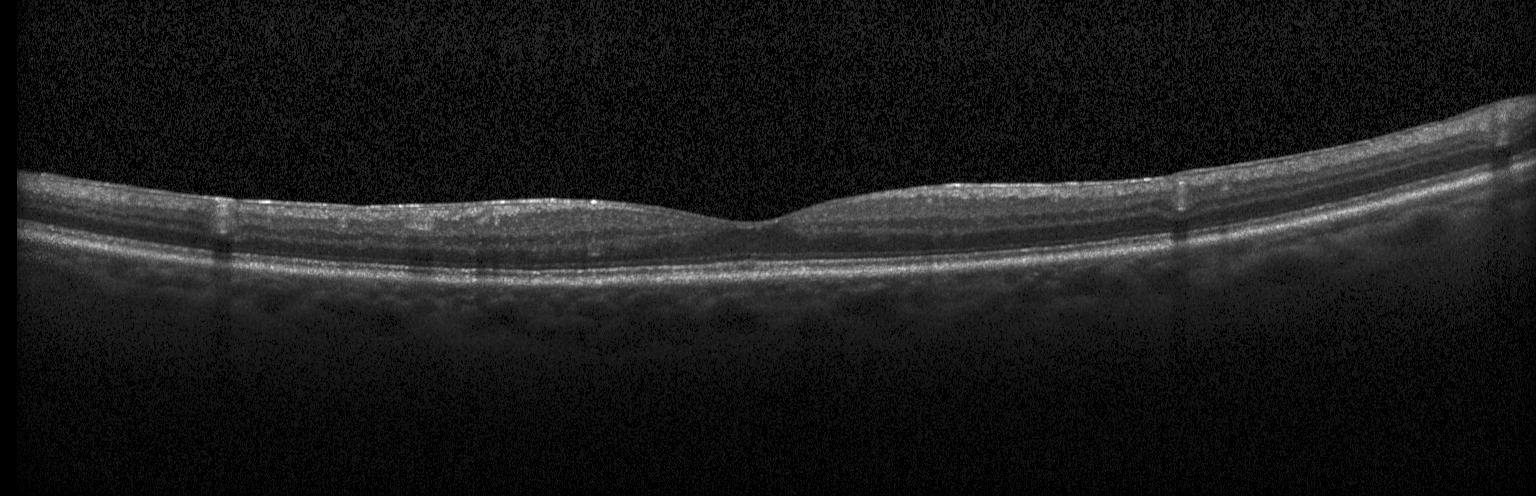
OCT finding: neither choroidal neovascularization, diabetic macular edema, nor drusen.